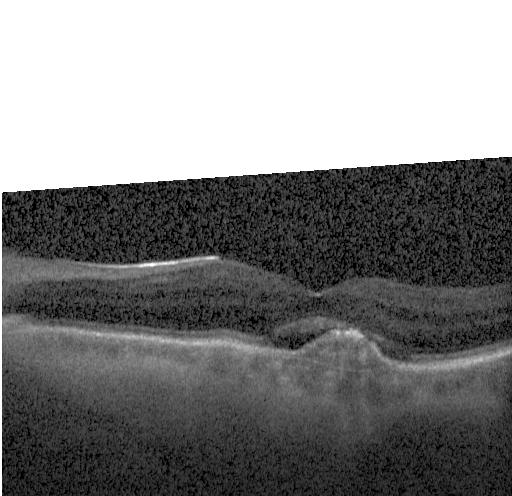

Impression: CNV.